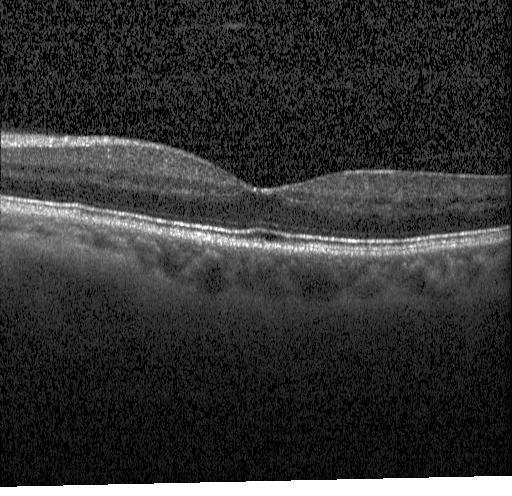

Fovea-centered, retinal OCT cross-section — OCT finding: no CNV, DME, or drusen.